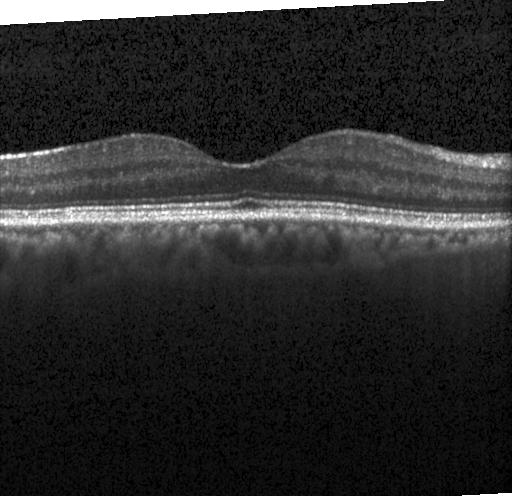 OCT B-scan. Impression: no choroidal neovascularization, diabetic macular edema, or drusen.